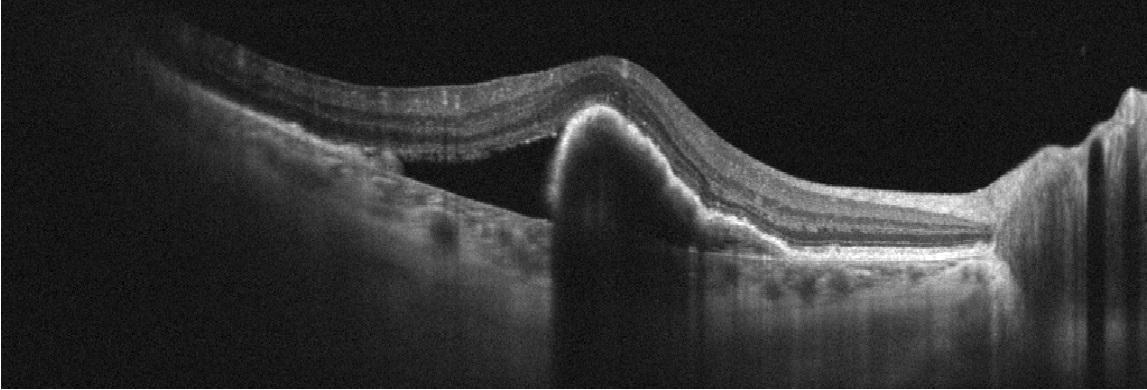

Acquired on an Optovue Avanti RTVue XR, OCT B-scan, fovea-centered.
Diagnosis: AMD.